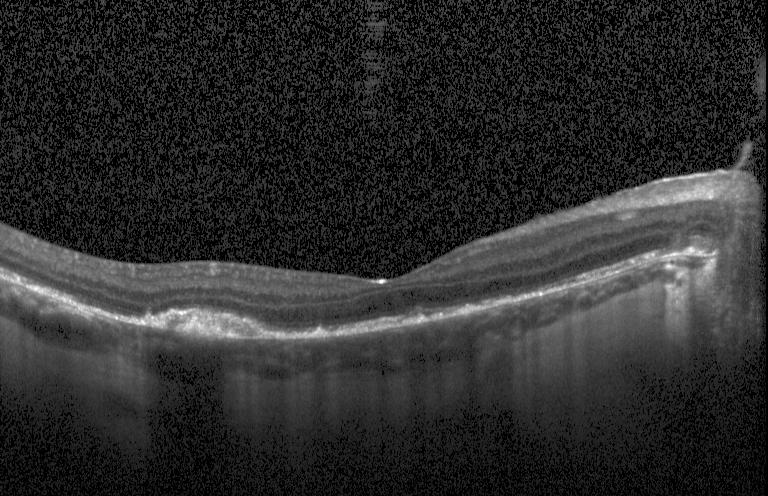
OCT B-scan; instrument: Heidelberg Spectralis; centered on the fovea.
Impression: choroidal neovascularization.